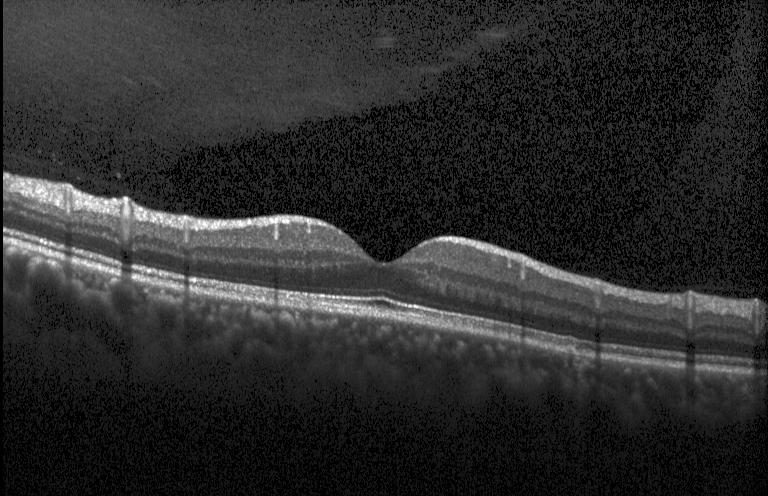 Diagnosis: no evidence of choroidal neovascularization, diabetic macular edema, or drusen.